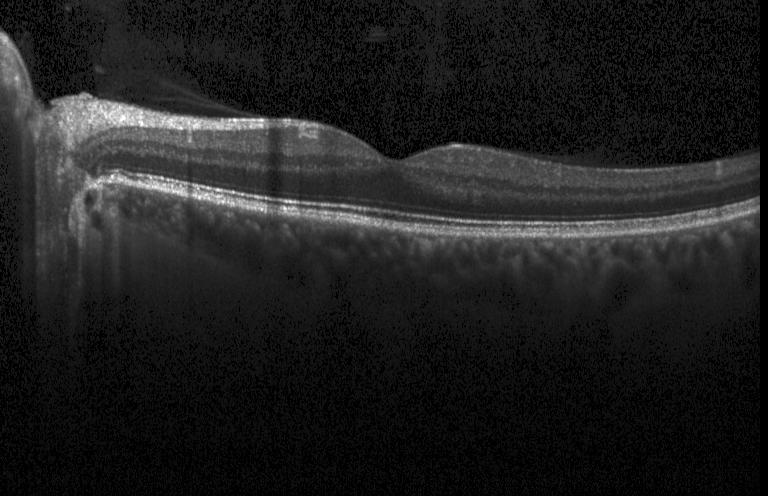
Retinal OCT cross-section.
Impression: no evidence of CNV, DME, or drusen.